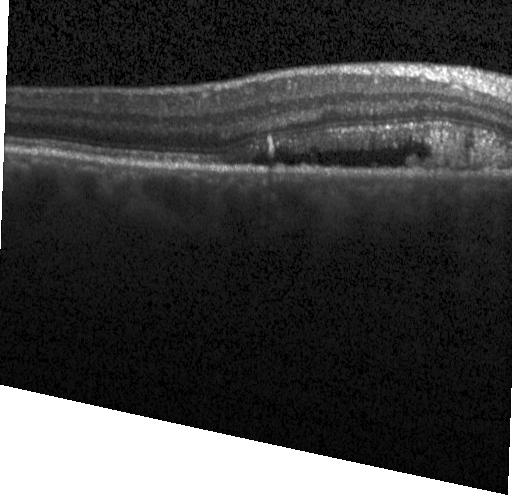
Impression: choroidal neovascularization (CNV).